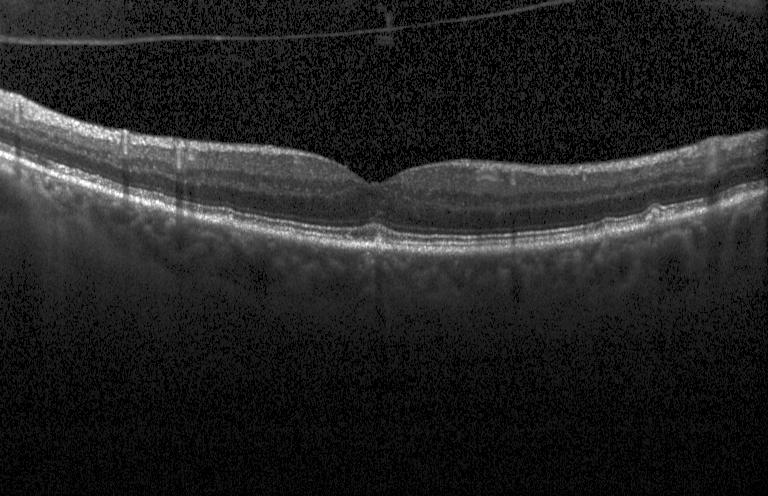 SD-OCT · OCT line scan.
Diagnosis: drusen.